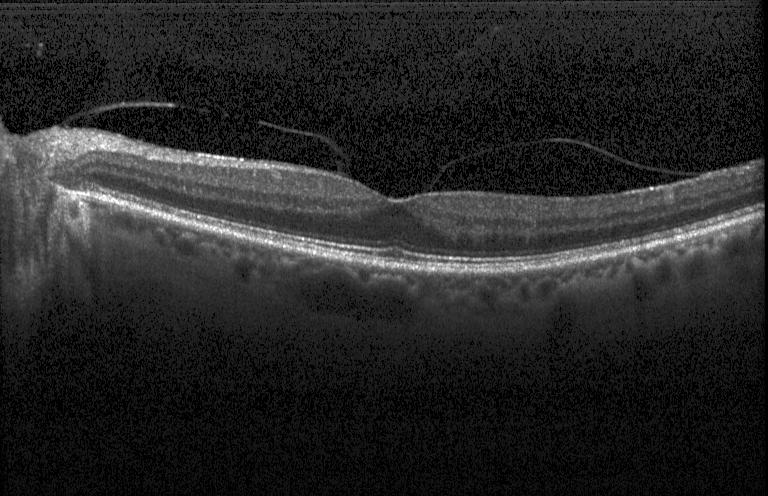
Horizontal scan through the fovea; optical coherence tomography scan; spectral-domain OCT. Impression: neither CNV, DME, nor drusen.